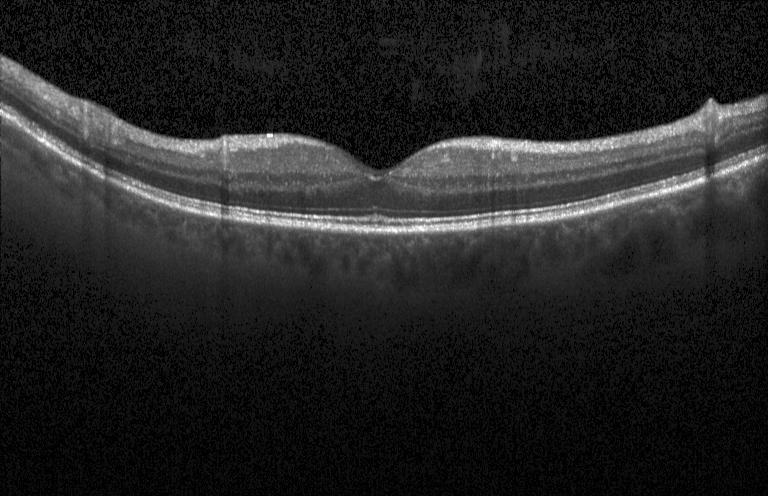

Retinal OCT cross-section showing no evidence of CNV, DME, or drusen.